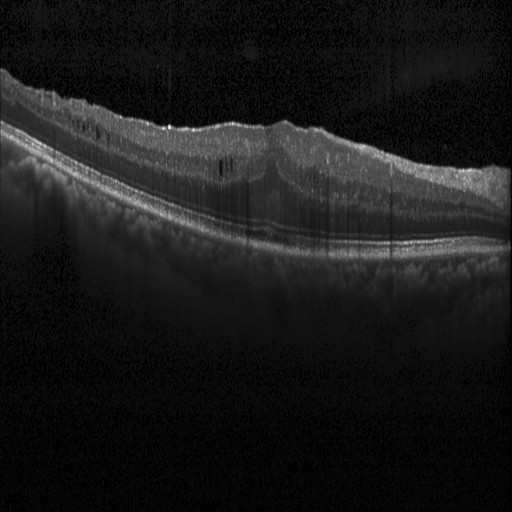 Through the macula · Heidelberg Spectralis OCT system · SD-OCT · retinal OCT B-scan — The scan shows diabetic macular edema.